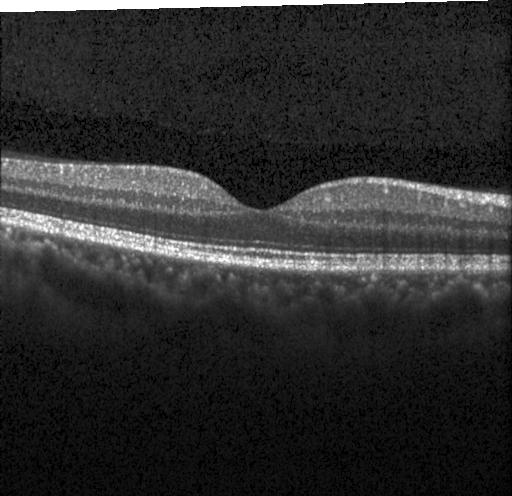 Acquired on a Heidelberg Spectralis. Optical coherence tomography scan
This B-scan demonstrates no choroidal neovascularization, no diabetic macular edema, and no drusen.